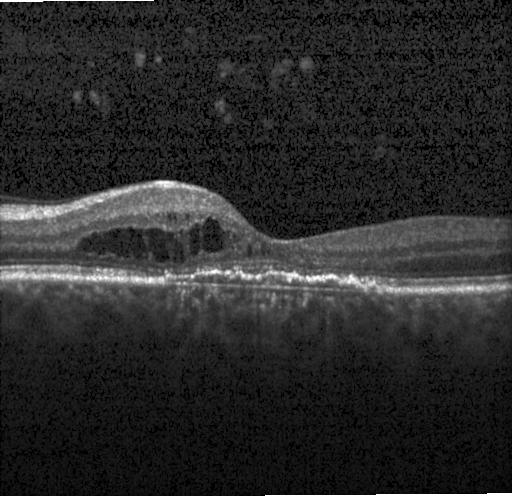 Retinal OCT cross-section
Choroidal neovascularization.